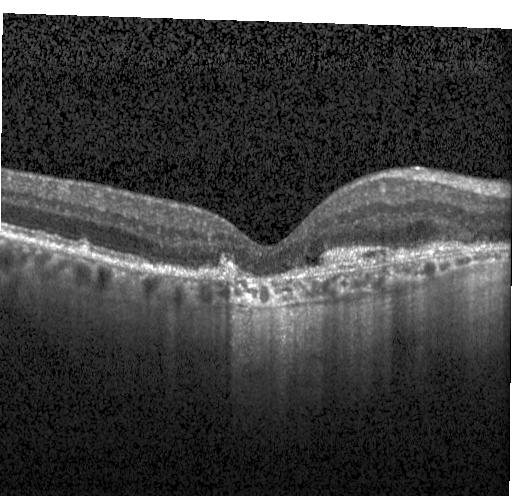

Finding: a choroidal neovascular membrane.